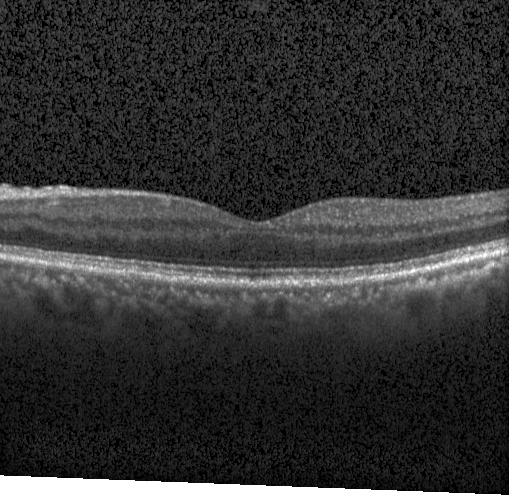 OCT line scan · fovea-centered · Heidelberg Spectralis · spectral-domain optical coherence tomography — Finding: neither CNV, DME, nor drusen.